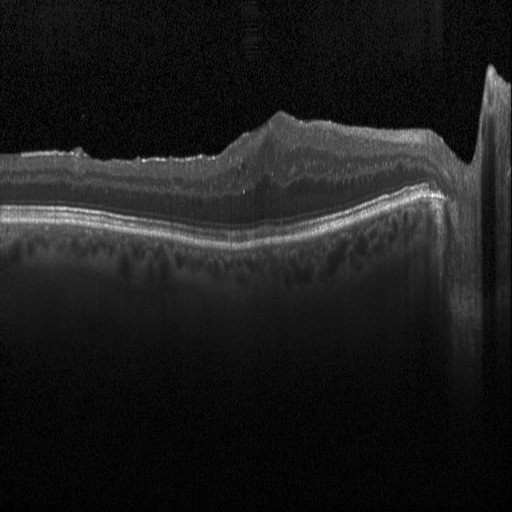

Heidelberg Spectralis OCT system, centered on the fovea, optical coherence tomography B-scan
DME.